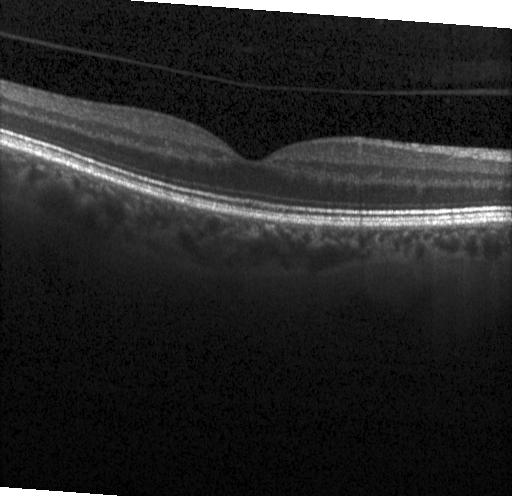
Spectral-domain OCT B-scan: neither CNV, DME, nor drusen.